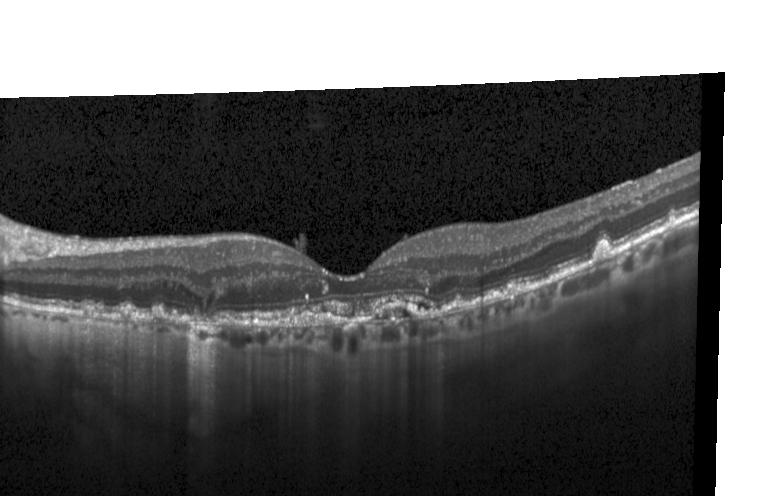
OCT B-scan · horizontal scan through the fovea · instrument: Heidelberg Spectralis · SD-OCT
A choroidal neovascular membrane.